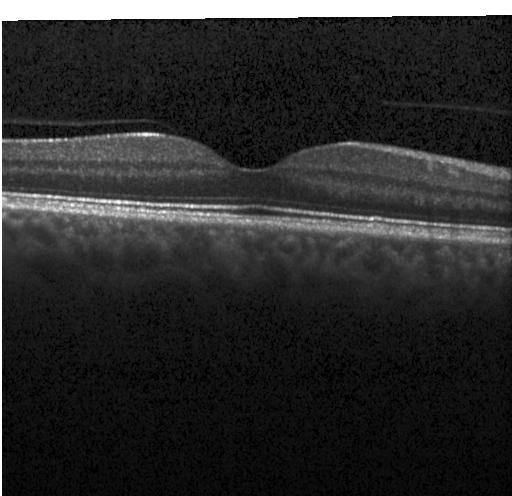 Spectral-domain optical coherence tomography · Heidelberg Spectralis · macular scan · retinal OCT B-scan. Finding: no choroidal neovascularization, diabetic macular edema, or drusen.